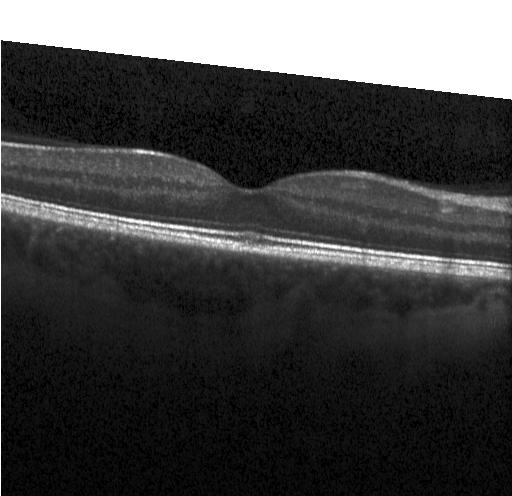

Finding: neither CNV, DME, nor drusen.